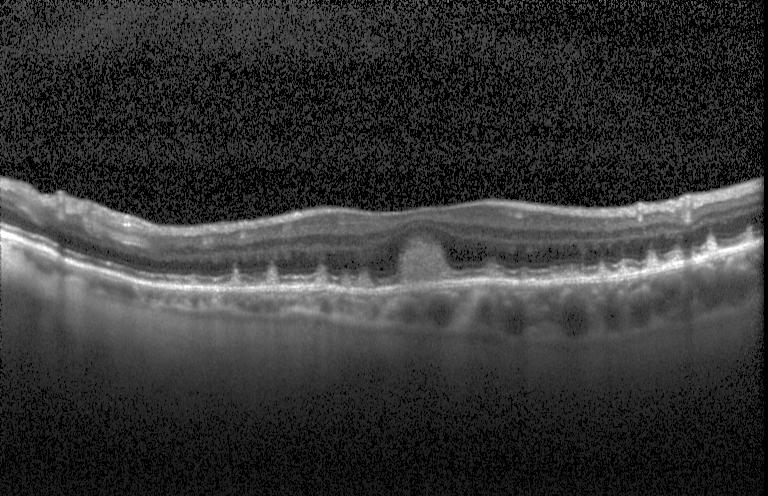
Spectral-domain OCT · optical coherence tomography scan. Diagnosis: a choroidal neovascular membrane.